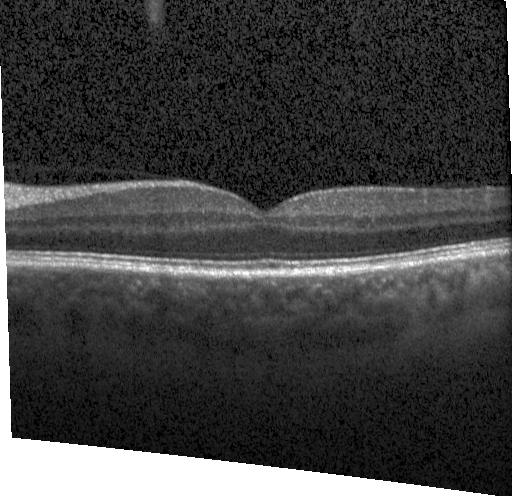
Finding: no CNV, no DME, and no drusen.